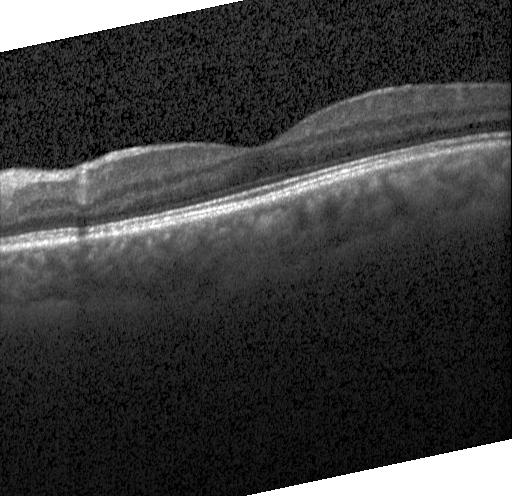

Horizontal scan through the fovea, OCT B-scan. OCT finding: no evidence of choroidal neovascularization, diabetic macular edema, or drusen.